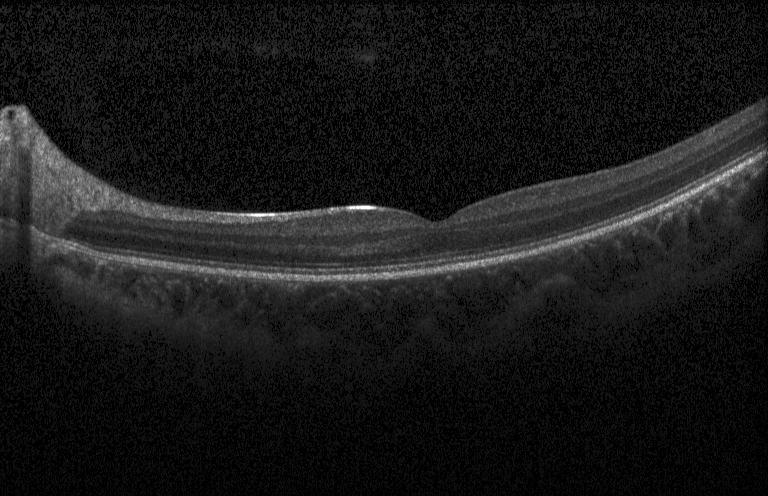 Finding: no evidence of choroidal neovascularization, diabetic macular edema, or drusen.